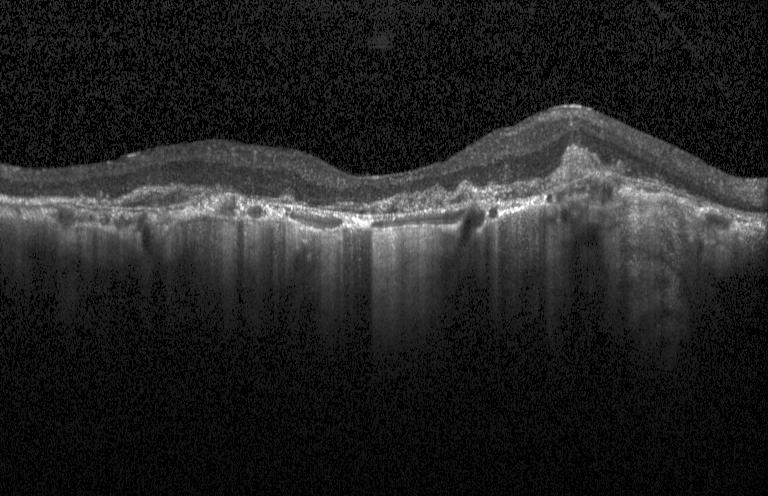

Macular OCT demonstrating choroidal neovascularization (CNV).